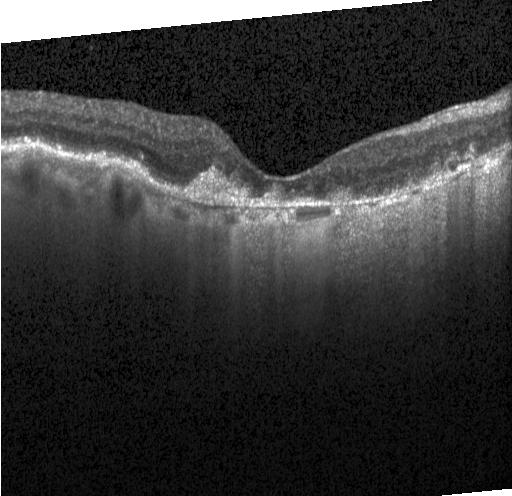

Optical coherence tomography scan — Macular OCT: CNV.